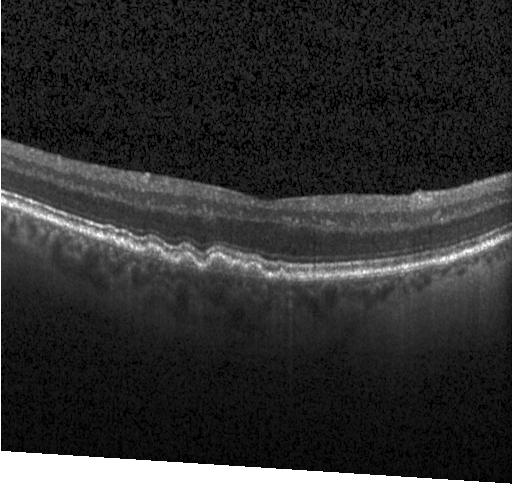 Macular OCT: drusen.